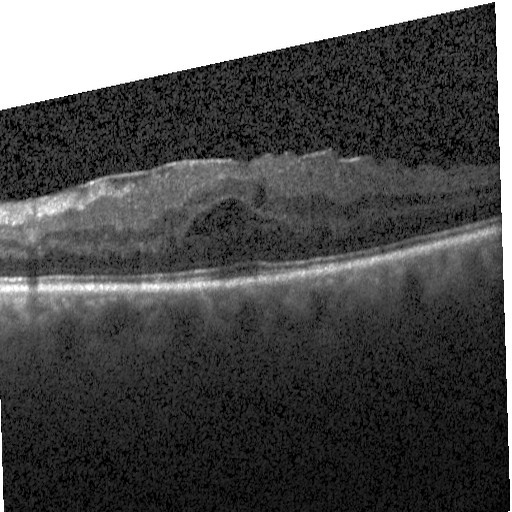
Optical coherence tomography scan · spectral-domain optical coherence tomography.
Diagnosis: DME.